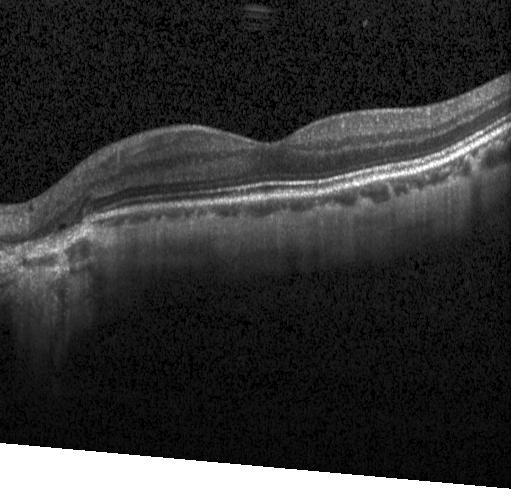 Spectral-domain OCT, Heidelberg Spectralis OCT system, retinal OCT cross-section. The scan shows no evidence of choroidal neovascularization, diabetic macular edema, or drusen.